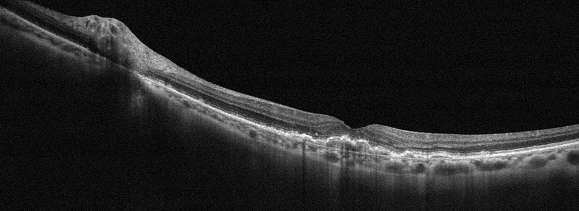

Left eye, retinal OCT B-scan.
Finding: AMD.